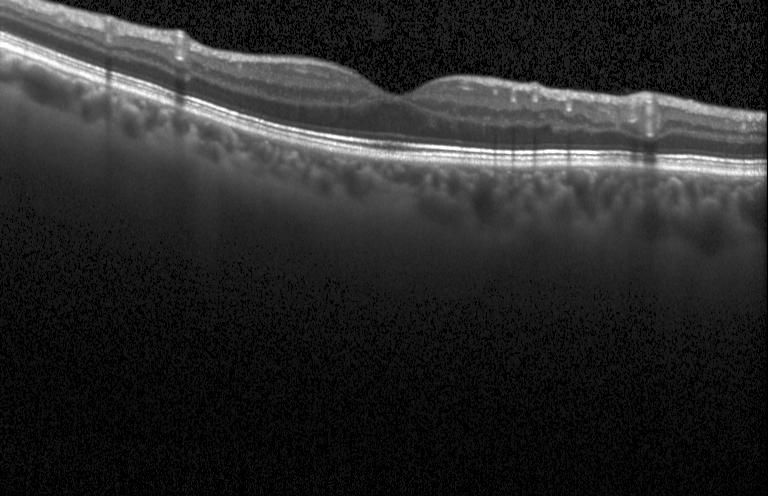
Optical coherence tomography scan. Heidelberg Spectralis OCT system
The scan shows no evidence of choroidal neovascularization, diabetic macular edema, or drusen.